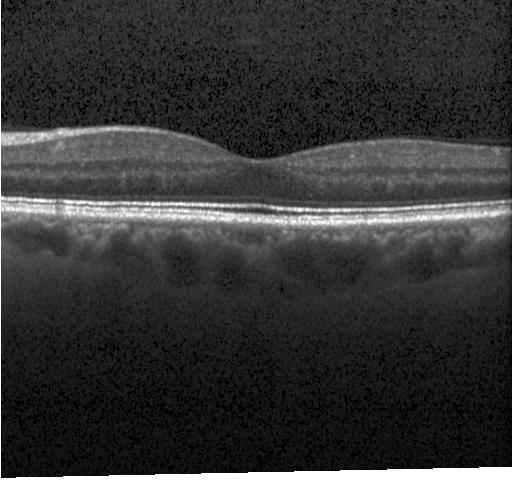 Spectral-domain OCT B-scan: neither CNV, DME, nor drusen.